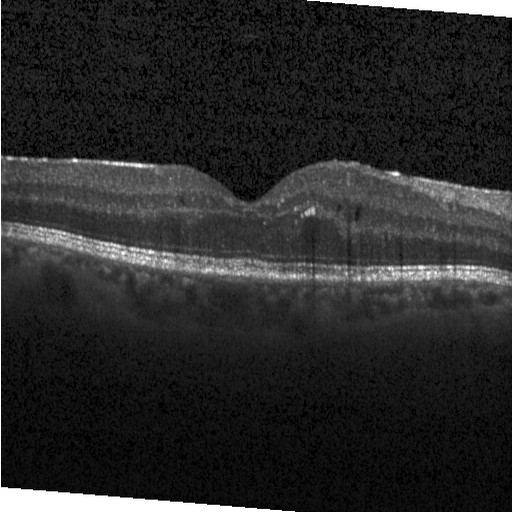 OCT line scan, centered on the fovea.
Macular OCT: DME.